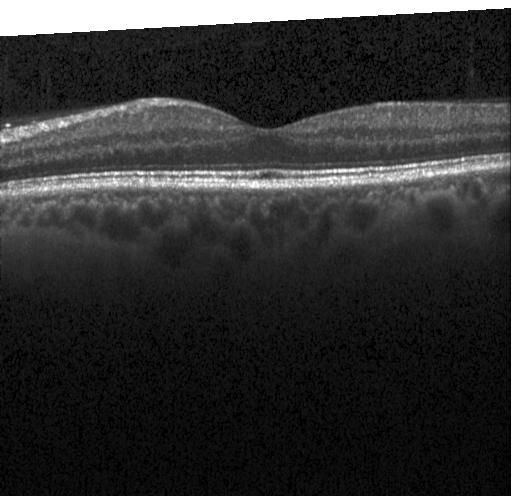

OCT line scan; acquired on a Heidelberg Spectralis. Neither CNV, DME, nor drusen.